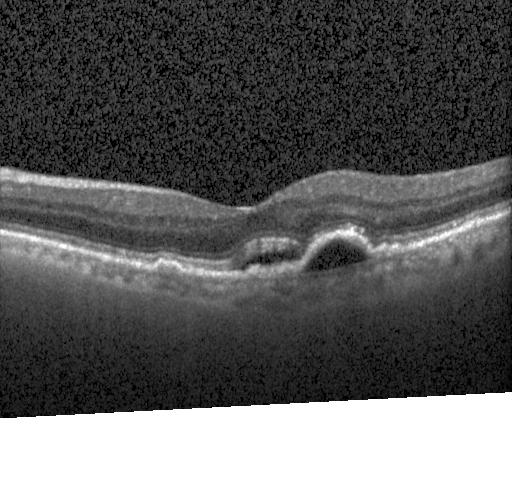
Acquired on a Heidelberg Spectralis; optical coherence tomography B-scan — Finding: a choroidal neovascular membrane.